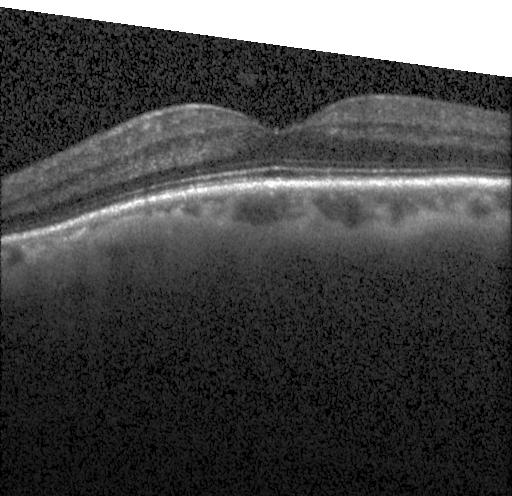 Heidelberg Spectralis OCT system. Optical coherence tomography scan. Horizontal scan through the fovea.
Dx: no evidence of CNV, DME, or drusen.